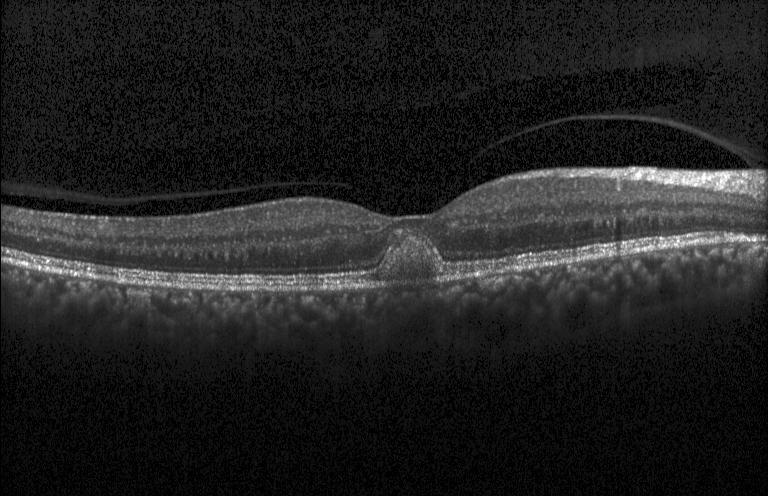
Macular scan; optical coherence tomography B-scan; Heidelberg Spectralis OCT system; spectral-domain OCT — This B-scan demonstrates choroidal neovascularization (CNV).